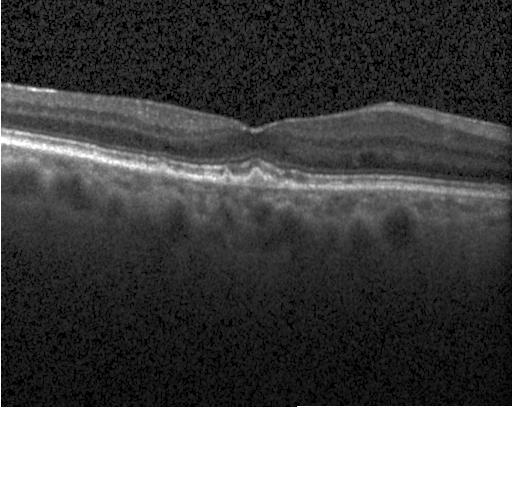 OCT line scan · spectral-domain OCT
Finding: drusen.